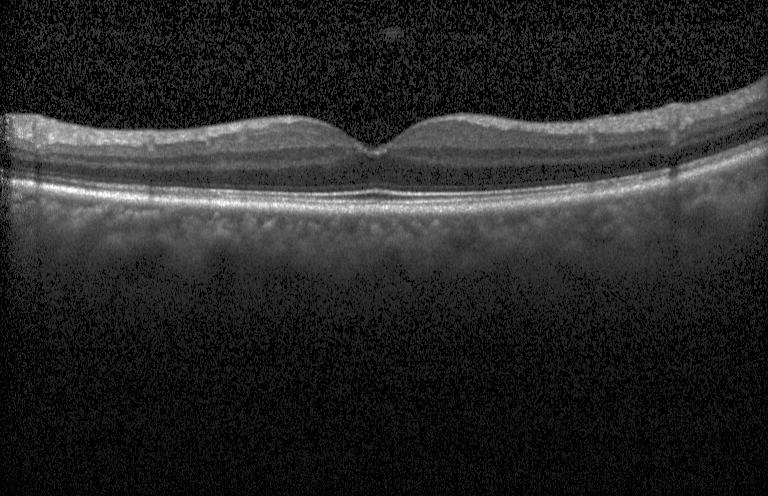 This B-scan demonstrates no evidence of CNV, DME, or drusen.